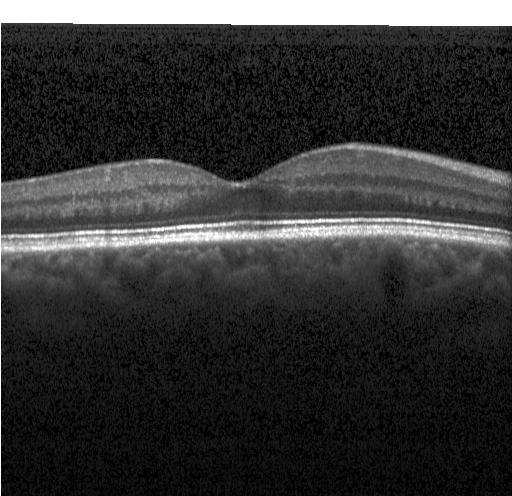

OCT B-scan · Heidelberg Spectralis — Dx: neither choroidal neovascularization, diabetic macular edema, nor drusen.